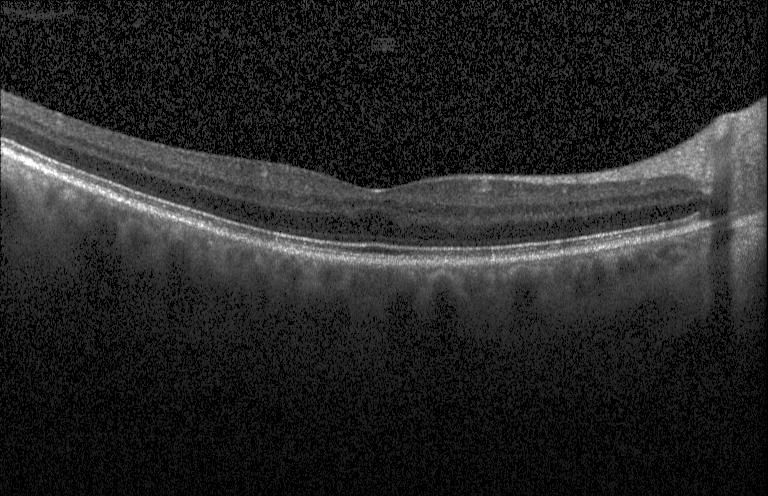 Spectral-domain OCT. OCT line scan — Impression: no choroidal neovascularization, diabetic macular edema, or drusen.